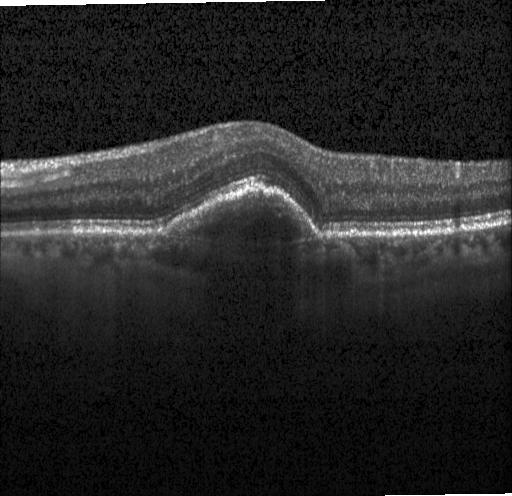 Acquired on a Heidelberg Spectralis. Retinal OCT B-scan.
Impression: choroidal neovascularization (CNV).